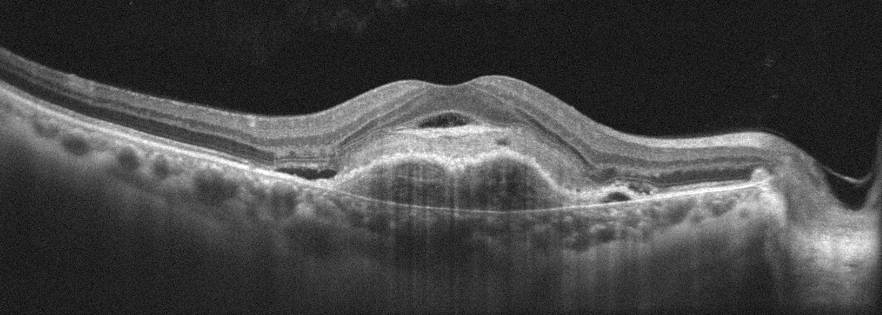

Through the macula, instrument: Optovue Avanti RTVue XR, right eye, retinal OCT cross-section — Finding: AMD.